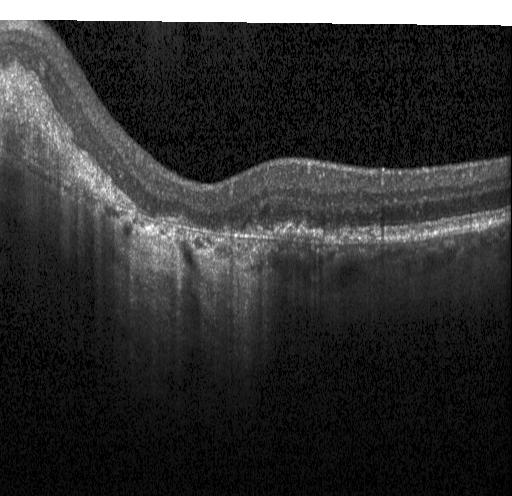

Spectral-domain optical coherence tomography. Fovea-centered. Retinal OCT cross-section. Heidelberg Spectralis OCT system — Finding: a choroidal neovascular membrane.